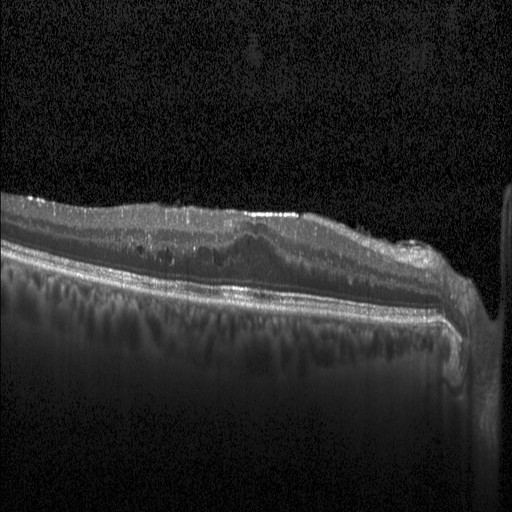
Assessment: diabetic macular edema.